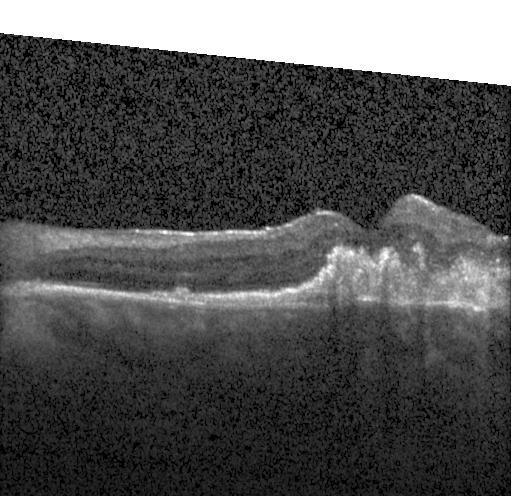

Retinal OCT cross-section · instrument: Heidelberg Spectralis — Macular OCT: a choroidal neovascular membrane.